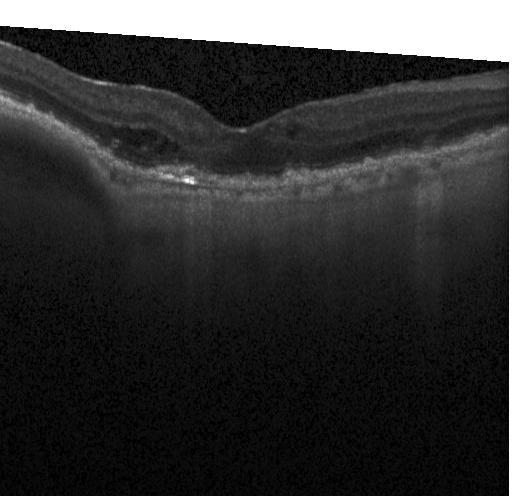
Diagnosis: choroidal neovascularization (CNV).